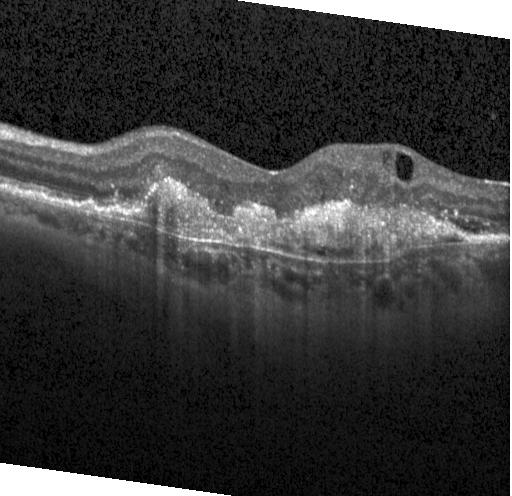 Spectral-domain OCT · Heidelberg Spectralis OCT system · OCT B-scan · centered on the fovea
Finding: a choroidal neovascular membrane.